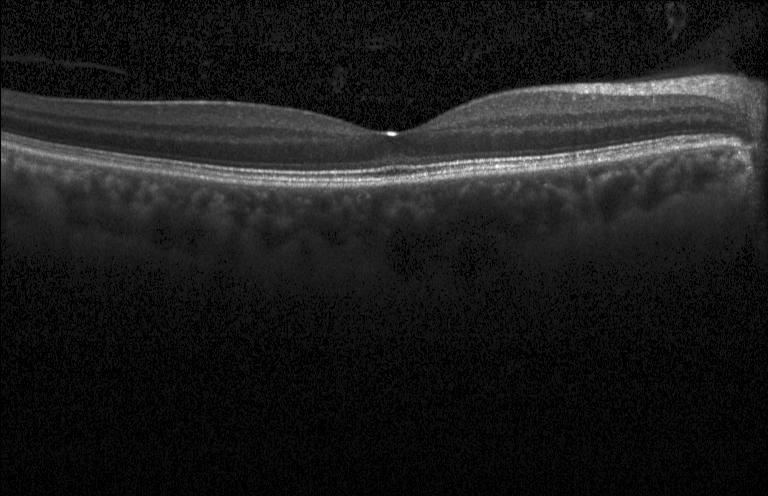
Spectral-domain OCT; OCT B-scan; acquired on a Heidelberg Spectralis; horizontal scan through the fovea
Finding: no choroidal neovascularization, no diabetic macular edema, and no drusen.